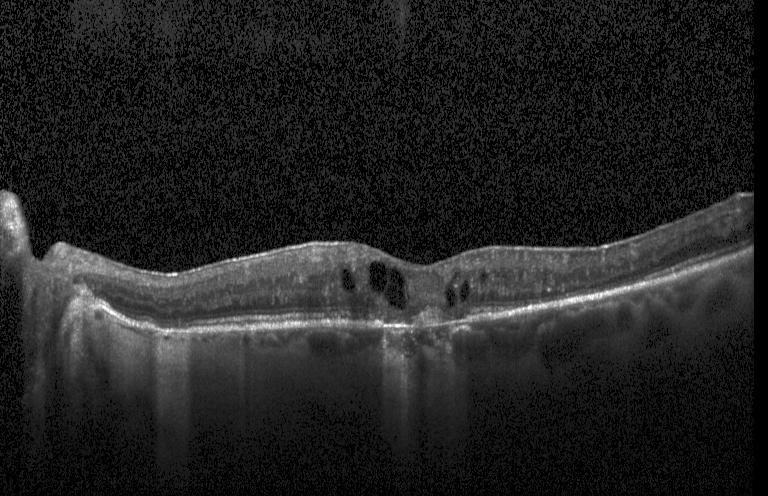

Finding: a choroidal neovascular membrane.